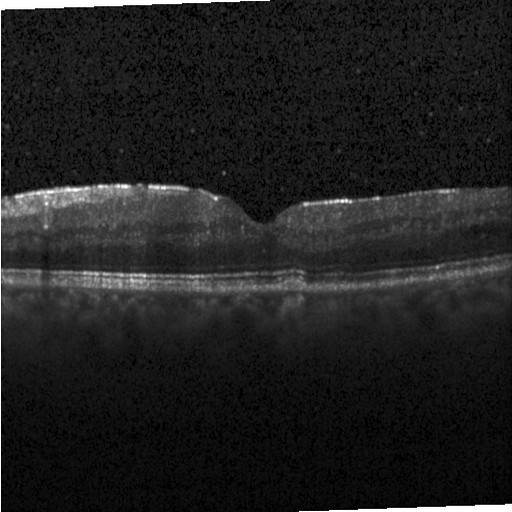 OCT finding: diabetic macular edema.